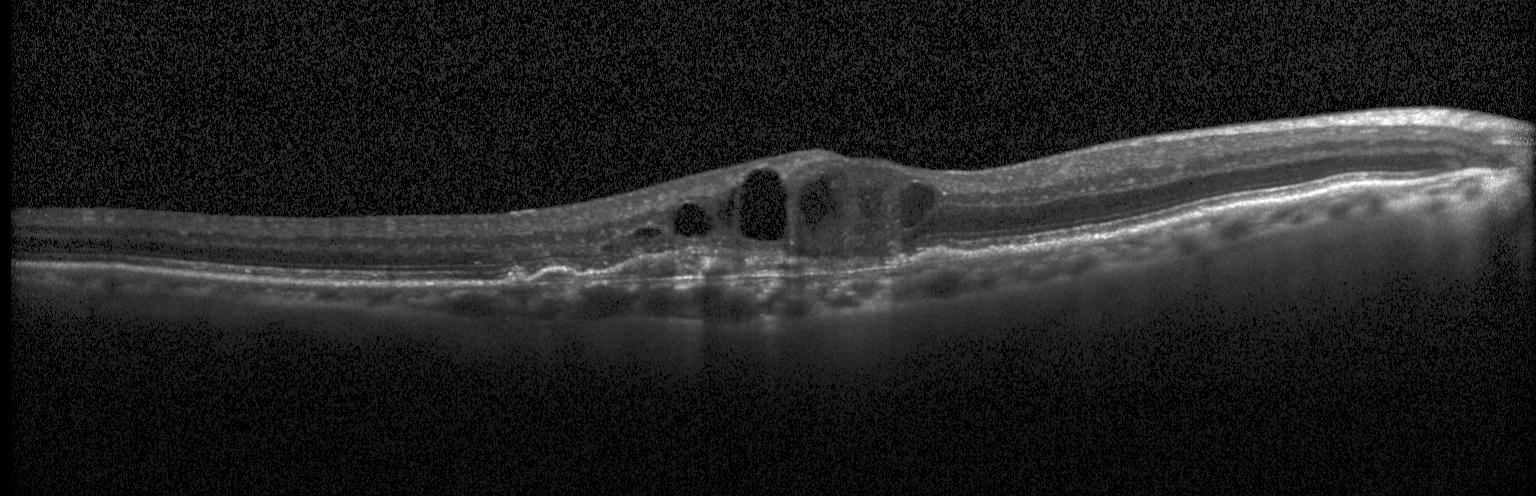
Impression: a choroidal neovascular membrane.